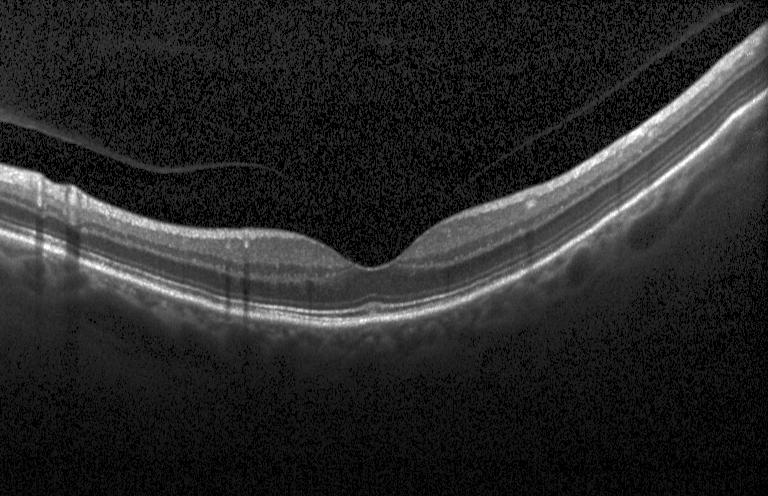 Optical coherence tomography scan. Spectral-domain optical coherence tomography. Through the macula. Acquired on a Heidelberg Spectralis
Assessment: no evidence of CNV, DME, or drusen.